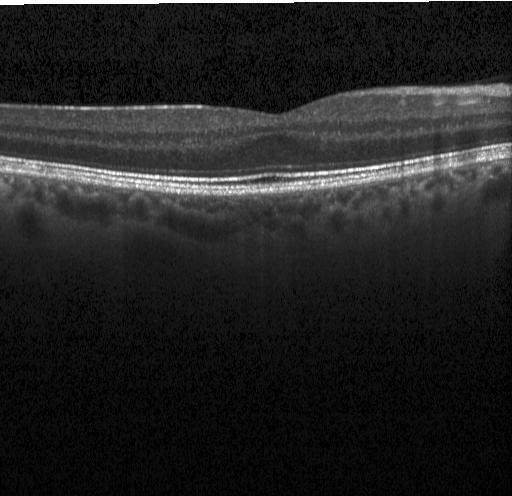 OCT line scan. Spectral-domain optical coherence tomography. Through the macula
Finding: no choroidal neovascularization, no diabetic macular edema, and no drusen.